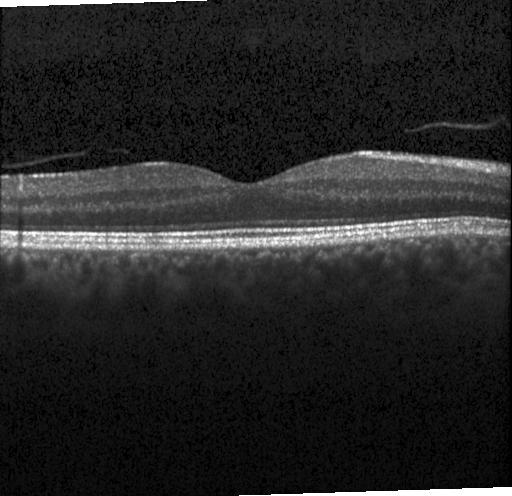
Spectral-domain OCT. Instrument: Heidelberg Spectralis. Optical coherence tomography scan.
OCT finding: neither choroidal neovascularization, diabetic macular edema, nor drusen.